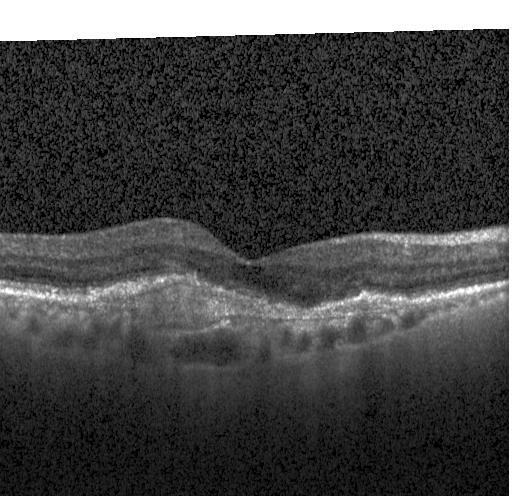 Retinal OCT B-scan — Assessment: choroidal neovascularization (CNV).